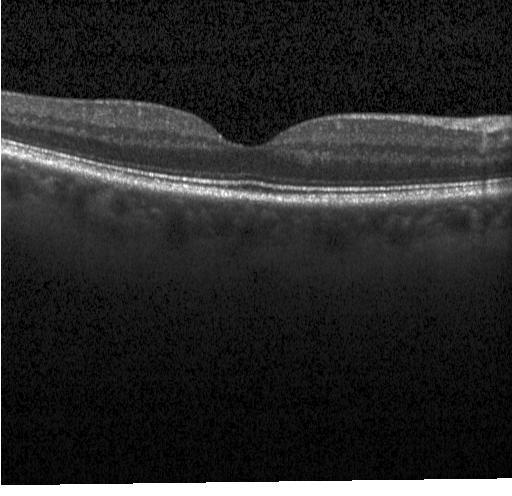

Macular OCT demonstrating neither choroidal neovascularization, diabetic macular edema, nor drusen.